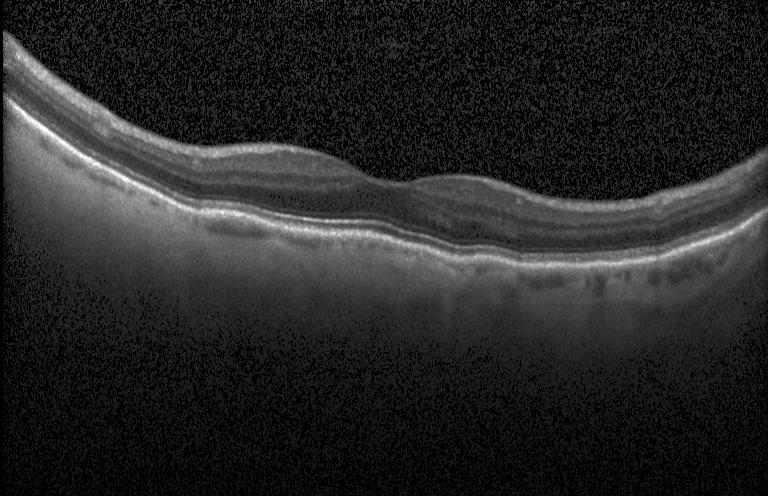
Optical coherence tomography scan; centered on the fovea.
Diagnosis: no evidence of CNV, DME, or drusen.